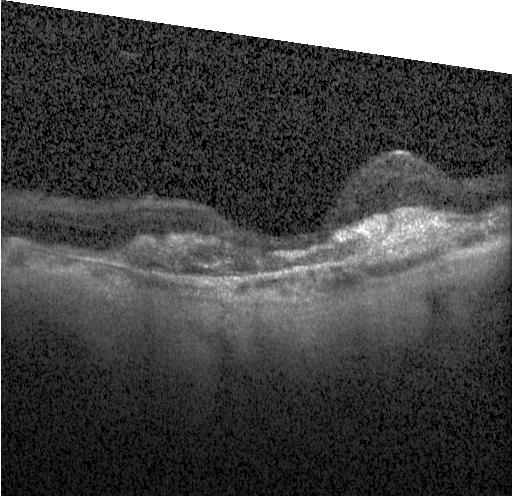
Impression: choroidal neovascularization.